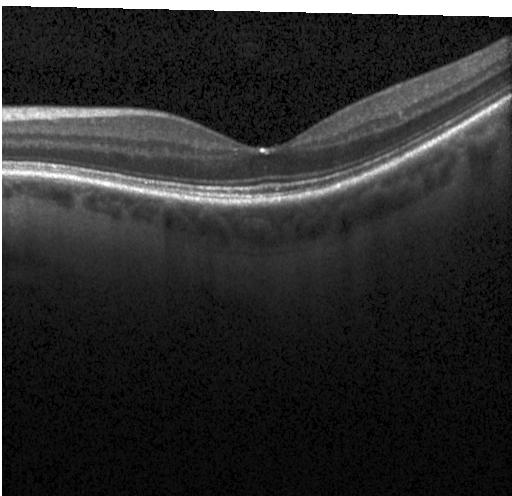 Heidelberg Spectralis OCT system · retinal OCT B-scan · spectral-domain OCT
Finding: neither choroidal neovascularization, diabetic macular edema, nor drusen.